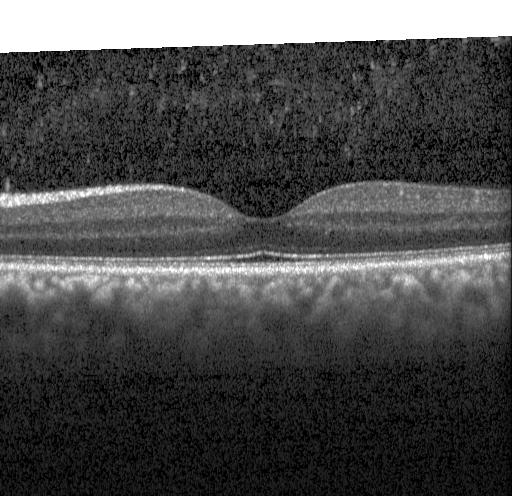
This B-scan demonstrates no CNV, no DME, and no drusen.